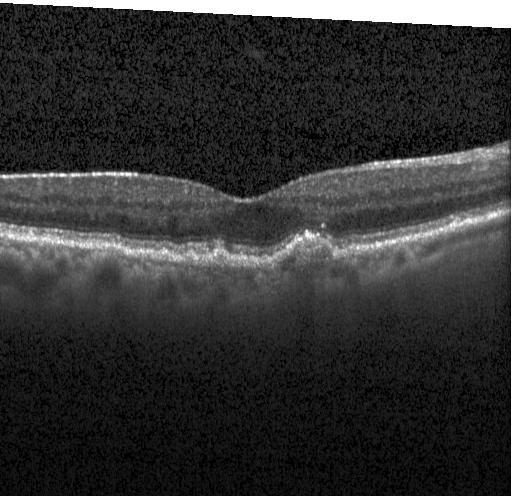

Spectral-domain OCT. Retinal OCT cross-section. Centered on the fovea. Heidelberg Spectralis. Macular OCT: CNV.